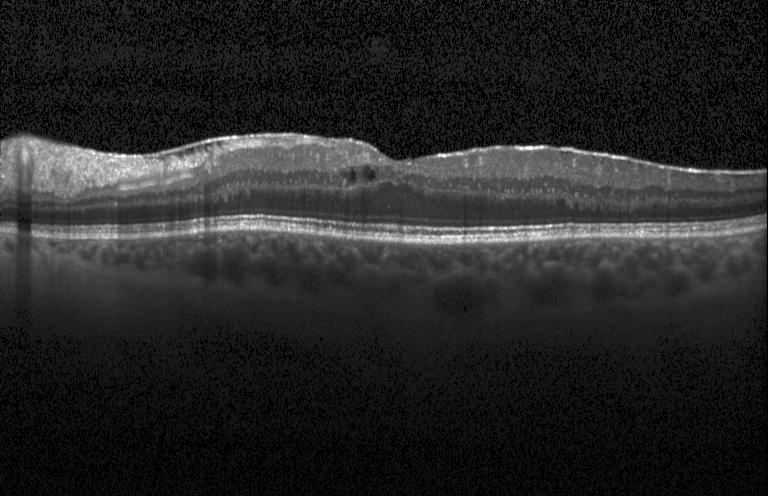 Retinal OCT B-scan. Macular scan. Heidelberg Spectralis OCT system.
The scan shows diabetic macular edema (DME).